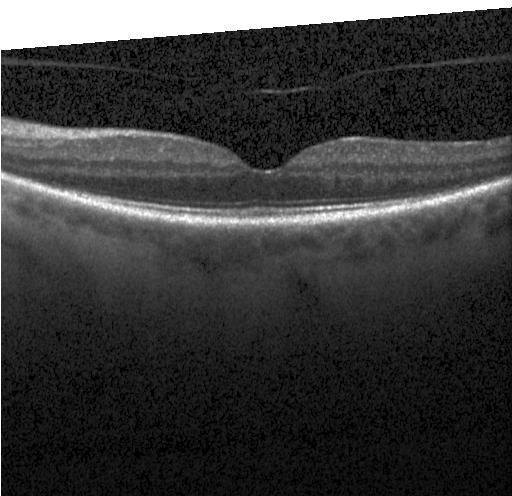 Acquired on a Heidelberg Spectralis · spectral-domain optical coherence tomography · OCT B-scan
Macular OCT: no choroidal neovascularization, no diabetic macular edema, and no drusen.